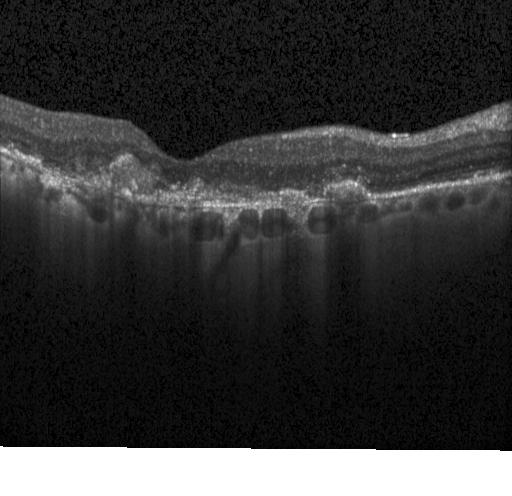 Retinal OCT cross-section
Impression: choroidal neovascularization.